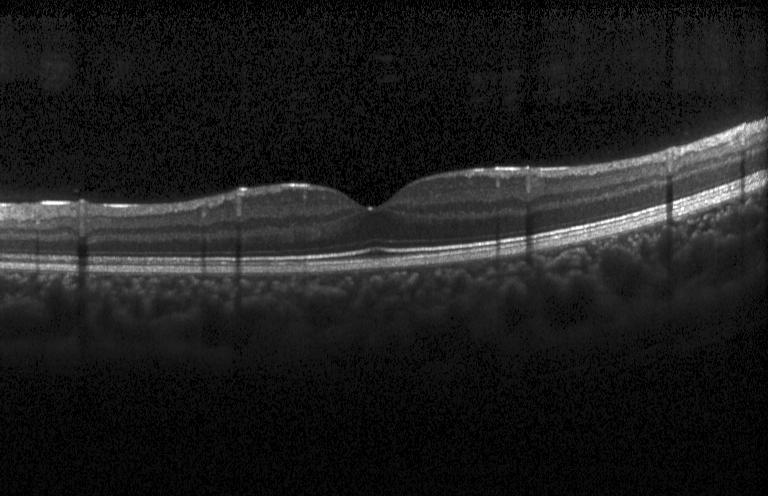

Spectral-domain optical coherence tomography. OCT line scan — The scan shows no choroidal neovascularization, no diabetic macular edema, and no drusen.